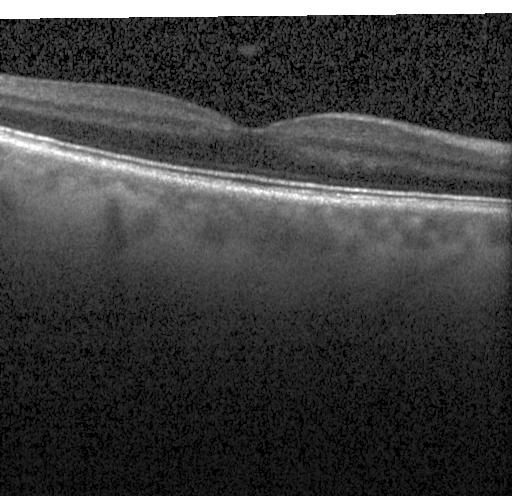

Instrument: Heidelberg Spectralis, optical coherence tomography B-scan.
Diagnosis: neither CNV, DME, nor drusen.